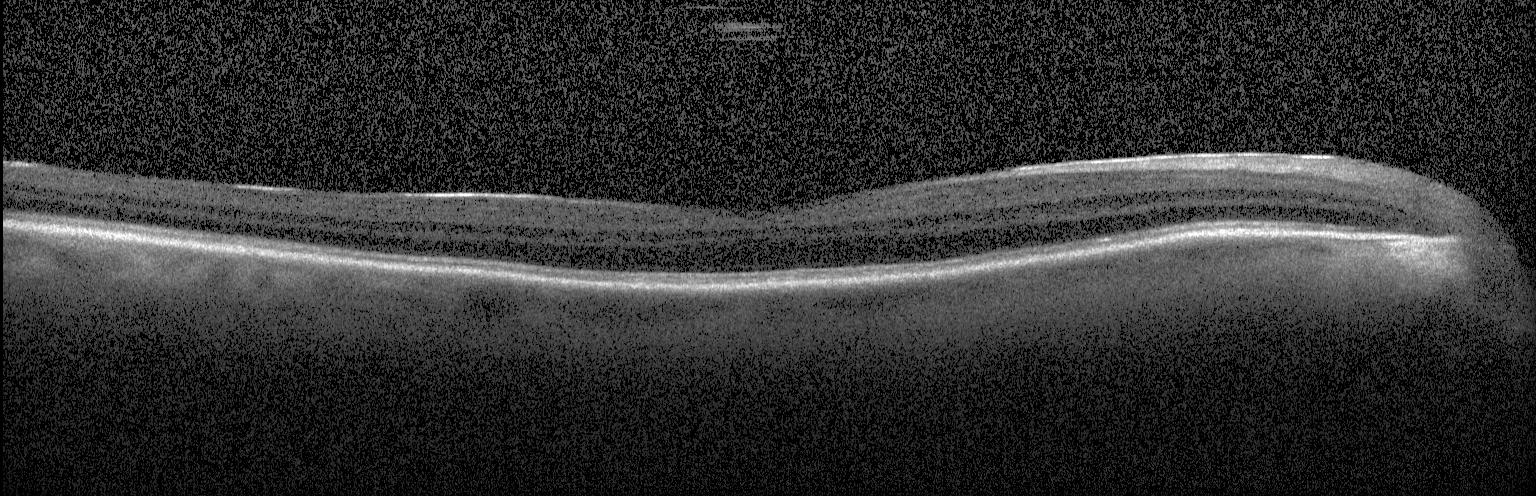 Spectral-domain optical coherence tomography · Heidelberg Spectralis · through the macula · retinal OCT cross-section — No evidence of choroidal neovascularization, diabetic macular edema, or drusen.